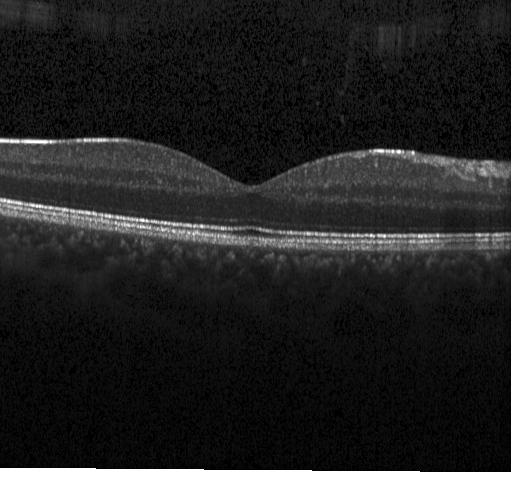

Diagnosis: no choroidal neovascularization, diabetic macular edema, or drusen.